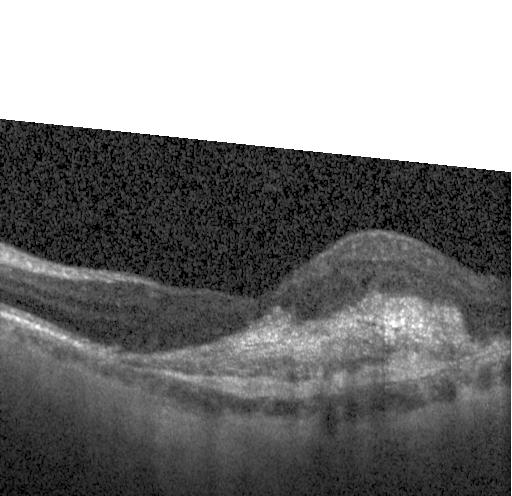

OCT finding: a choroidal neovascular membrane.